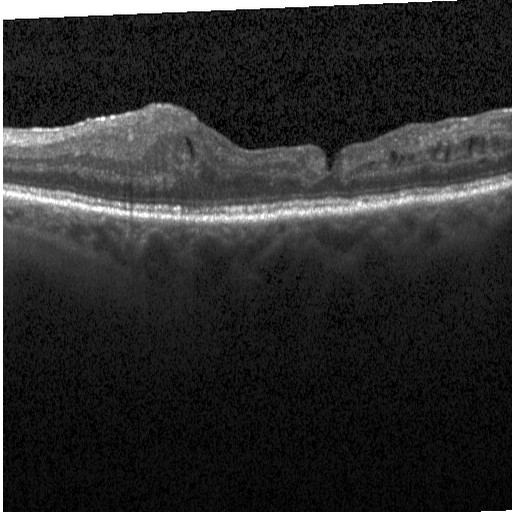

Through the macula; optical coherence tomography scan — Impression: diabetic macular edema.